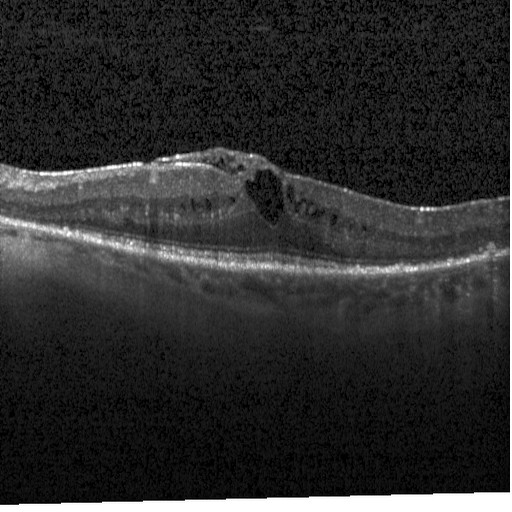
Dx: diabetic macular edema (DME).